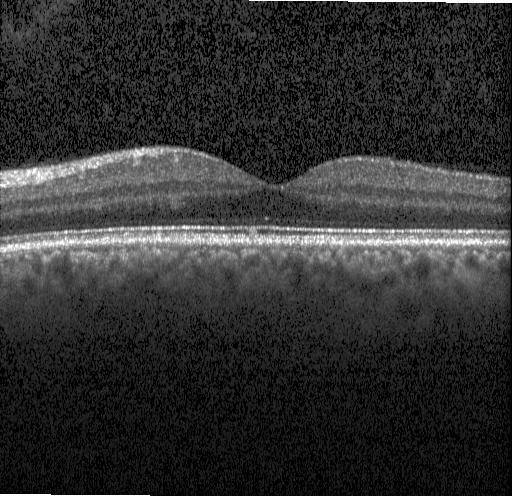 Macular OCT: no CNV, no DME, and no drusen.